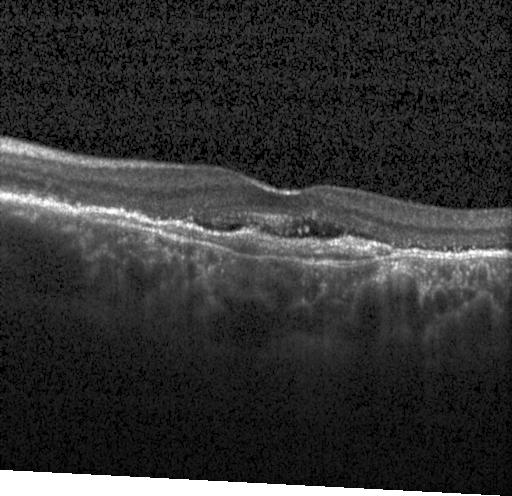

Retinal OCT B-scan · acquired on a Heidelberg Spectralis · through the macula · spectral-domain optical coherence tomography — The scan shows choroidal neovascularization (CNV).